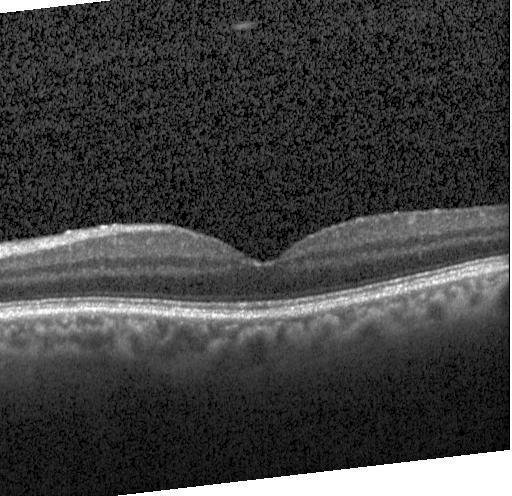

Impression: no evidence of CNV, DME, or drusen.